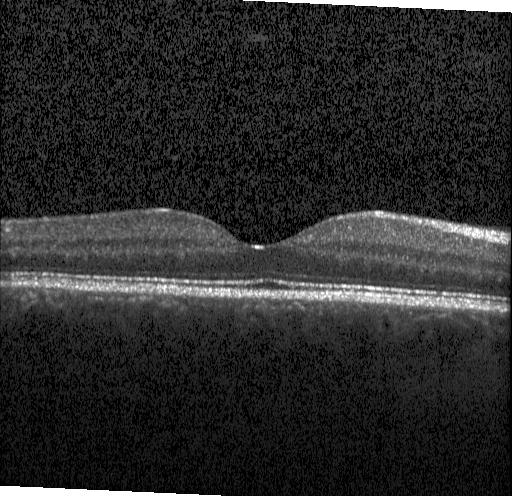

Instrument: Heidelberg Spectralis, spectral-domain optical coherence tomography, optical coherence tomography scan
The scan shows no choroidal neovascularization, diabetic macular edema, or drusen.